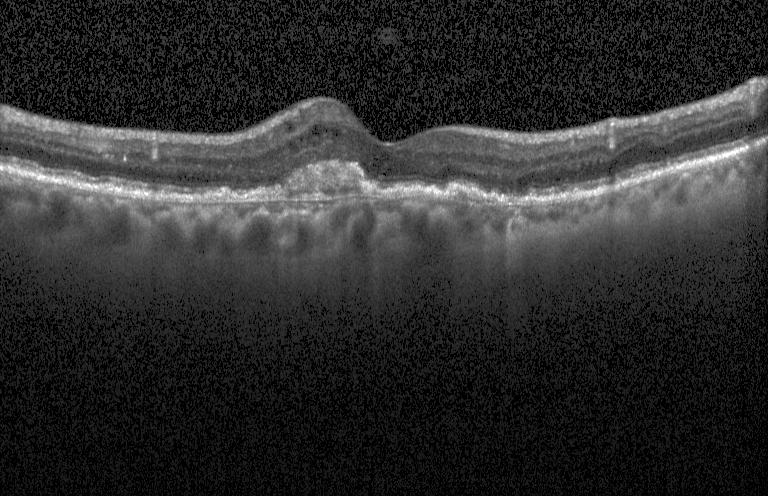

CNV.